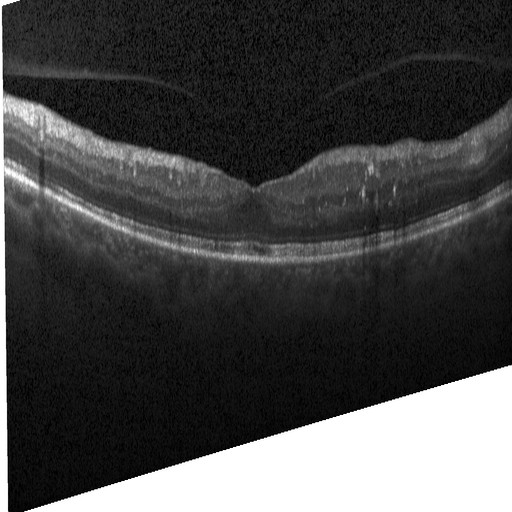 Fovea-centered. Acquired on a Heidelberg Spectralis. Optical coherence tomography scan.
Dx: DME.